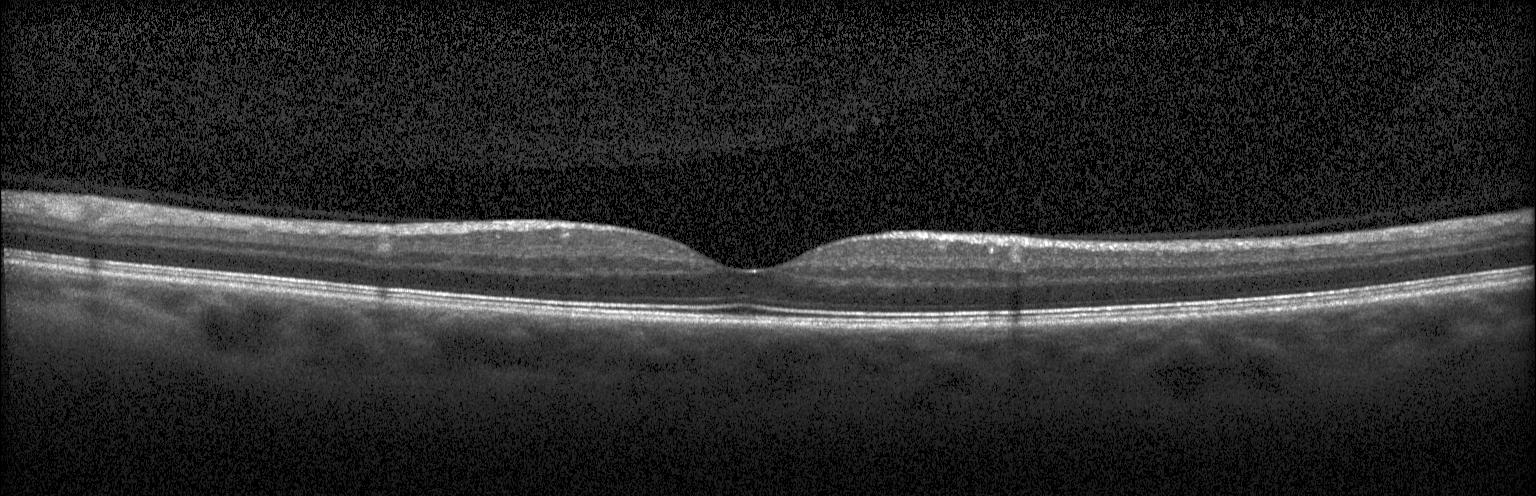

Retinal OCT cross-section showing neither CNV, DME, nor drusen.